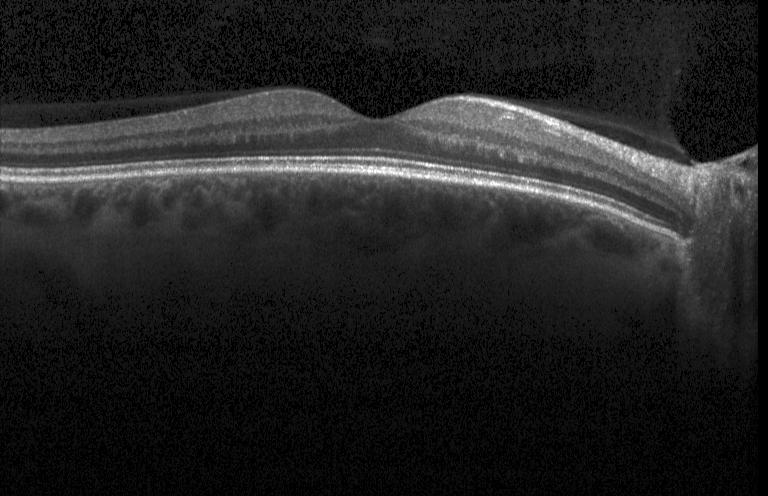

Diagnosis: no evidence of choroidal neovascularization, diabetic macular edema, or drusen.